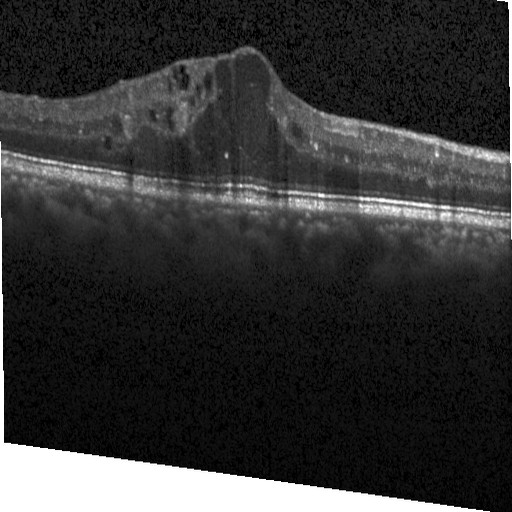

Retinal OCT cross-section showing diabetic macular edema (DME).